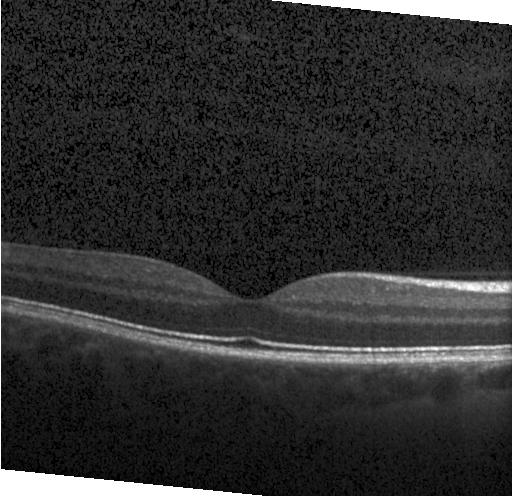 Assessment: neither choroidal neovascularization, diabetic macular edema, nor drusen.